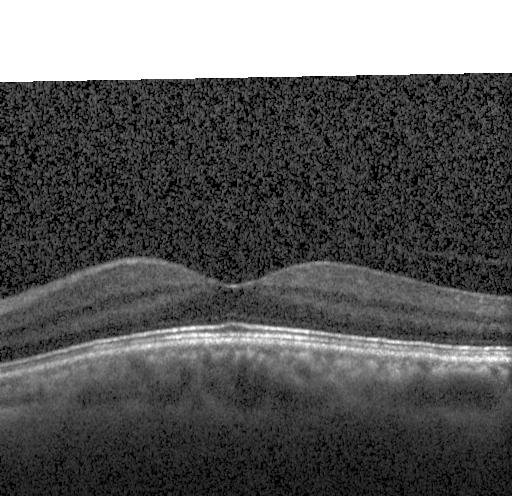
Retinal OCT B-scan; spectral-domain optical coherence tomography
OCT finding: neither CNV, DME, nor drusen.